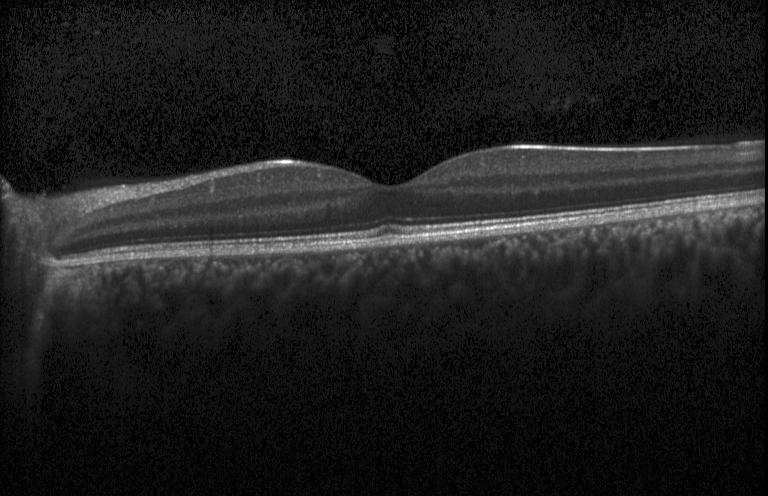

Diagnosis: no evidence of choroidal neovascularization, diabetic macular edema, or drusen.